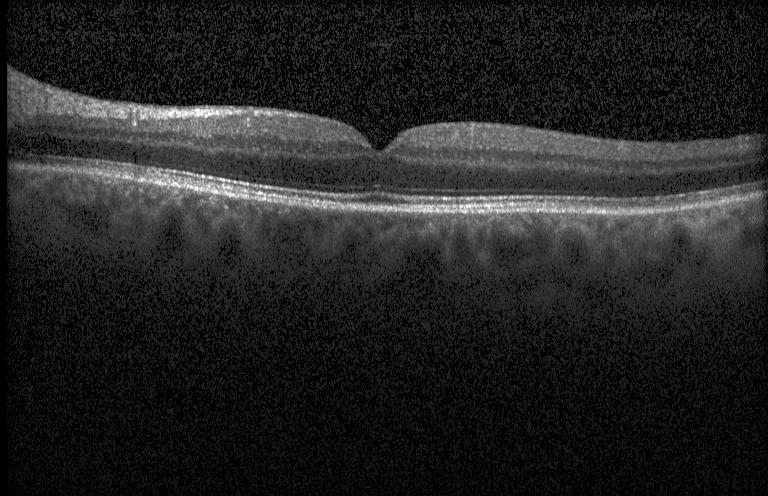
Dx: neither choroidal neovascularization, diabetic macular edema, nor drusen.